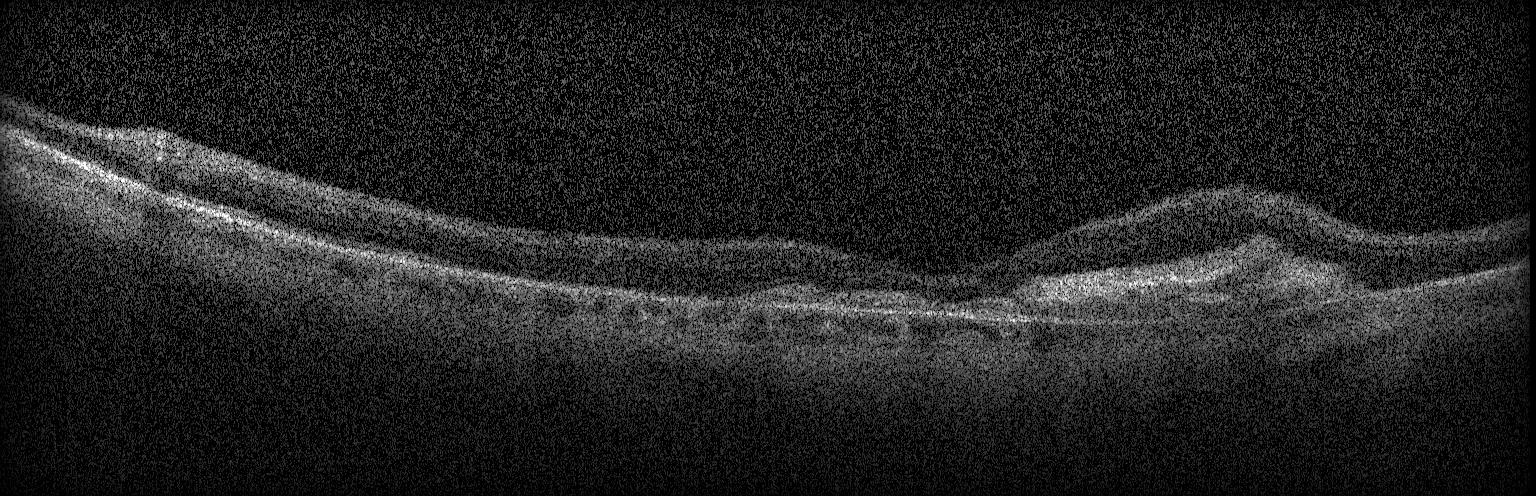

Assessment: a choroidal neovascular membrane.